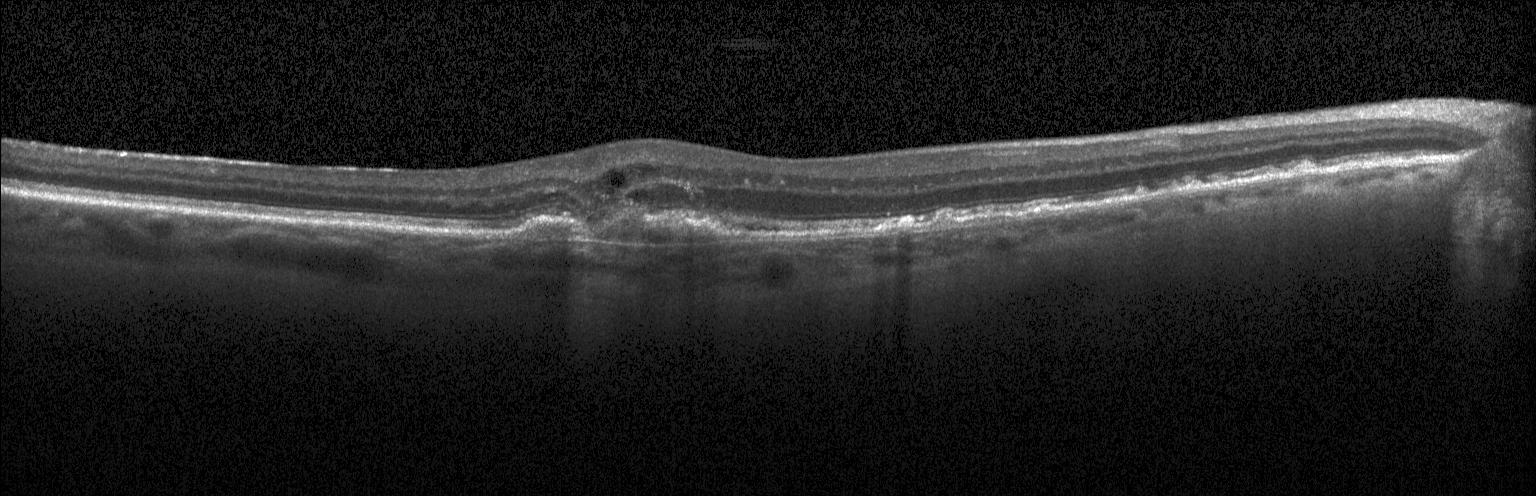 Fovea-centered. SD-OCT. OCT line scan. Heidelberg Spectralis.
OCT finding: a choroidal neovascular membrane.